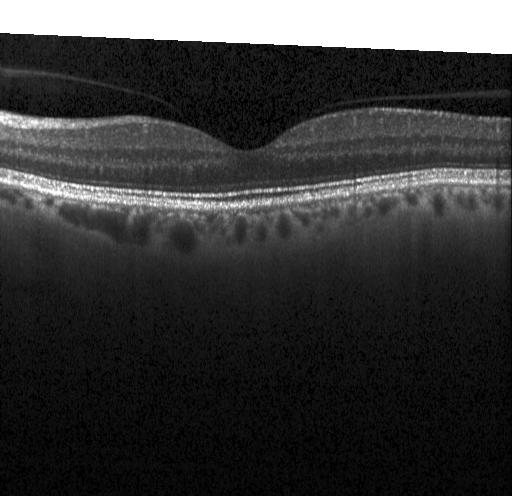

OCT line scan, centered on the fovea, SD-OCT.
Diagnosis: no choroidal neovascularization, diabetic macular edema, or drusen.